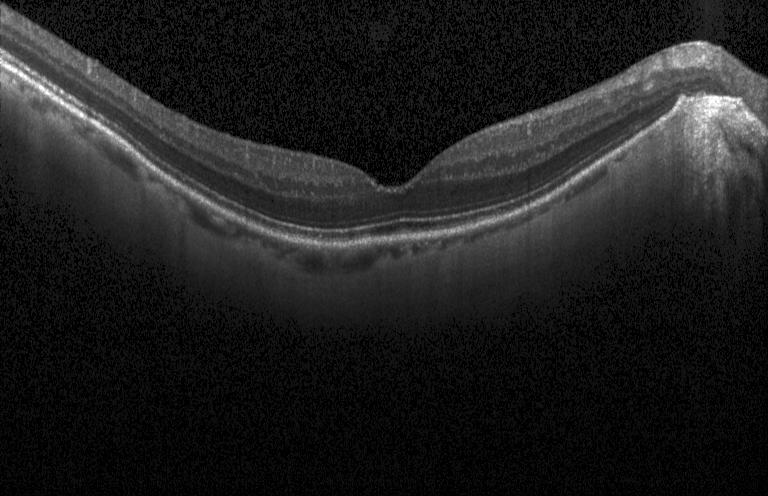

OCT scan showing no CNV, DME, or drusen.